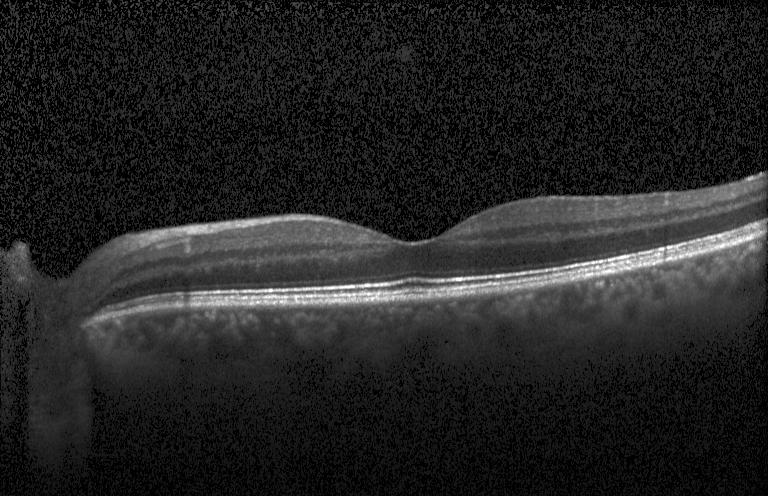
Heidelberg Spectralis · SD-OCT · macular scan · OCT B-scan.
The scan shows no choroidal neovascularization, diabetic macular edema, or drusen.